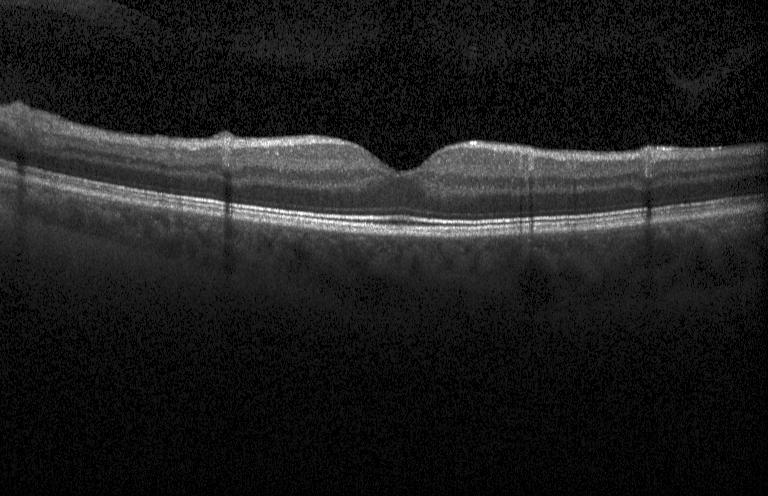 Macular OCT demonstrating neither CNV, DME, nor drusen.